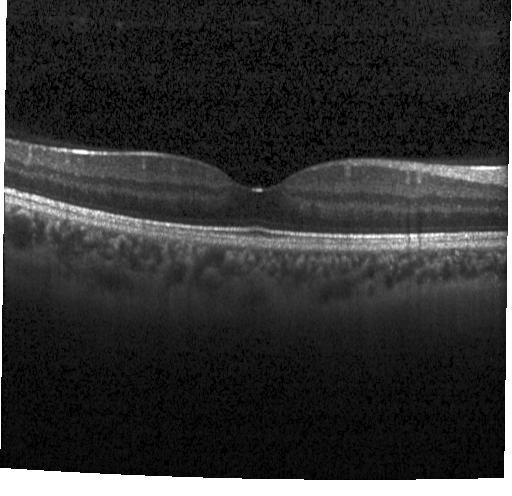 Retinal OCT B-scan · spectral-domain optical coherence tomography.
This B-scan demonstrates neither CNV, DME, nor drusen.